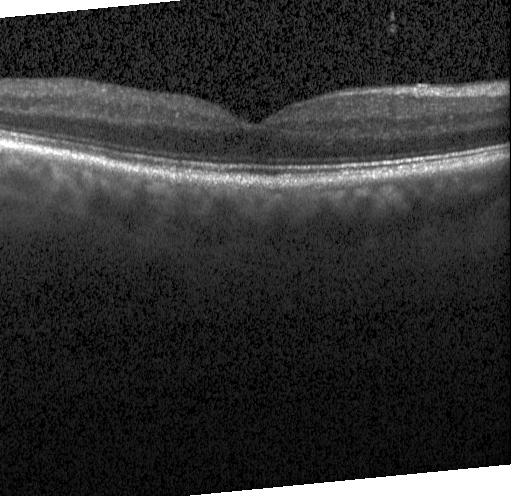

Optical coherence tomography B-scan — OCT finding: neither CNV, DME, nor drusen.